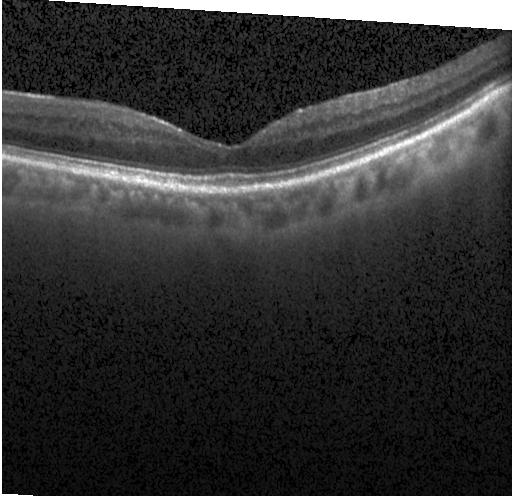
Acquired on a Heidelberg Spectralis, horizontal scan through the fovea, optical coherence tomography B-scan, spectral-domain OCT
OCT finding: no evidence of choroidal neovascularization, diabetic macular edema, or drusen.